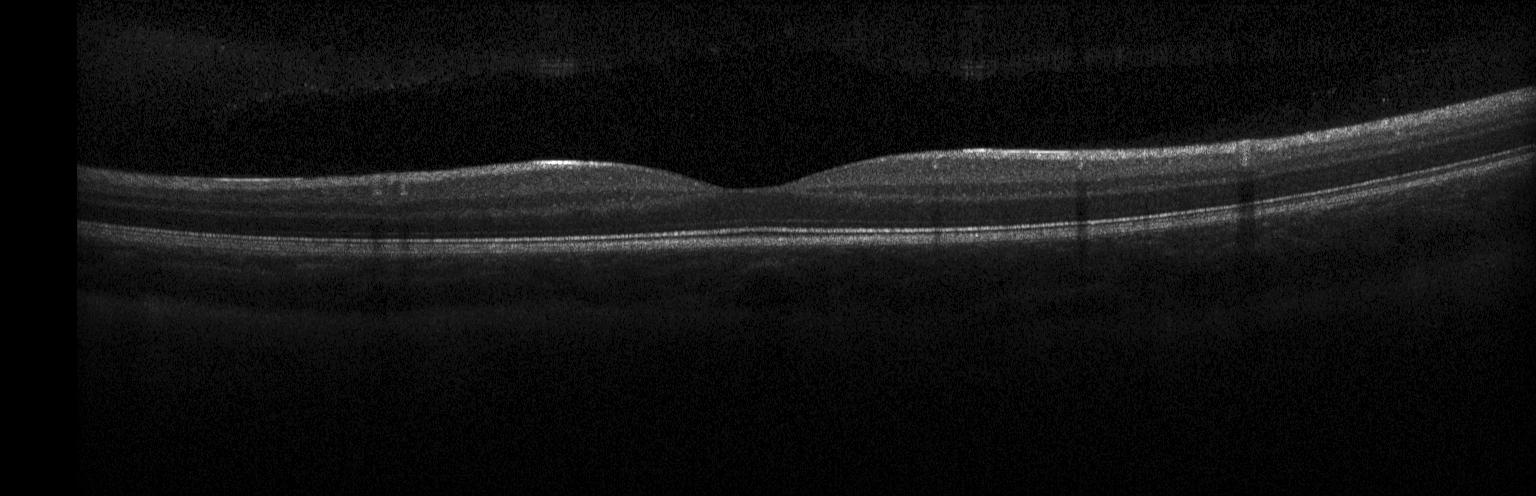
Retinal OCT B-scan, Heidelberg Spectralis. Finding: no choroidal neovascularization, no diabetic macular edema, and no drusen.